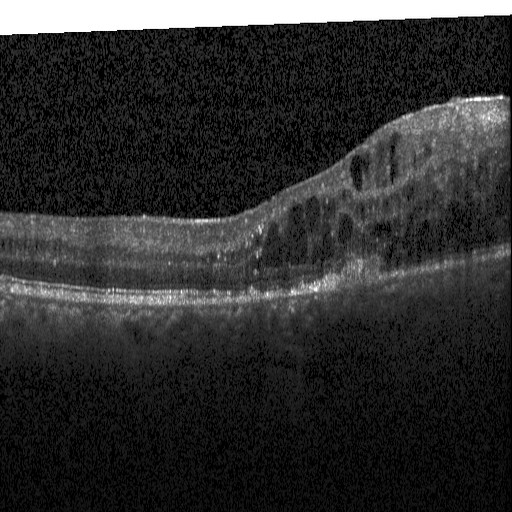

Retinal OCT B-scan. OCT finding: DME.